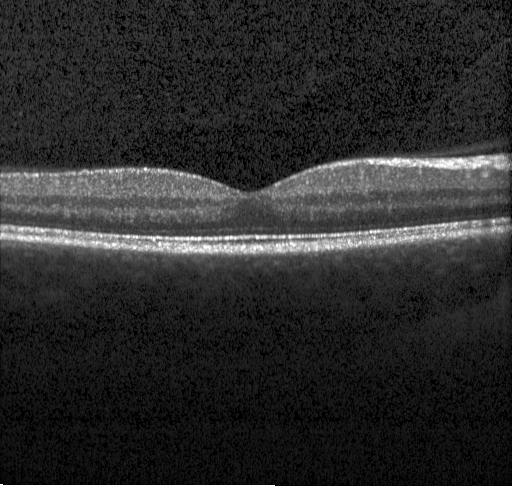
No choroidal neovascularization, diabetic macular edema, or drusen.